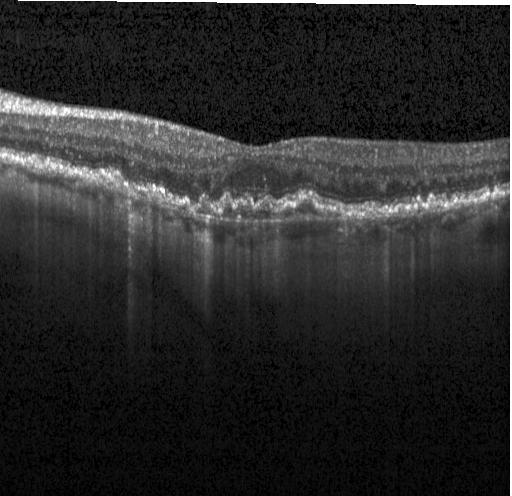

Assessment: a choroidal neovascular membrane.